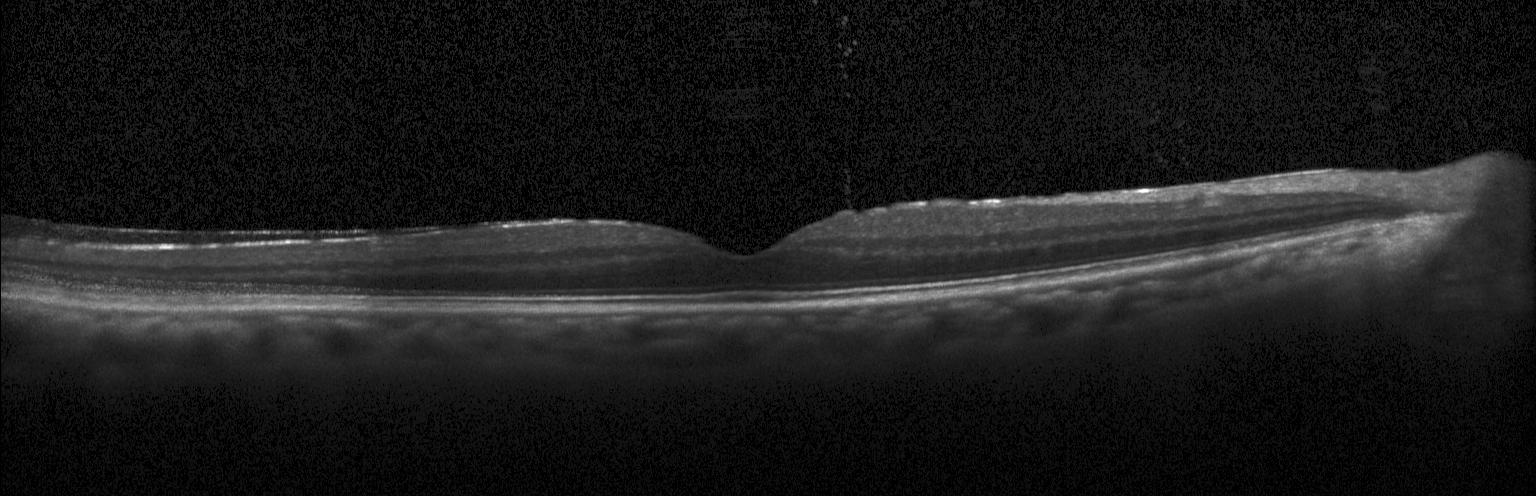

OCT B-scan. Impression: neither choroidal neovascularization, diabetic macular edema, nor drusen.